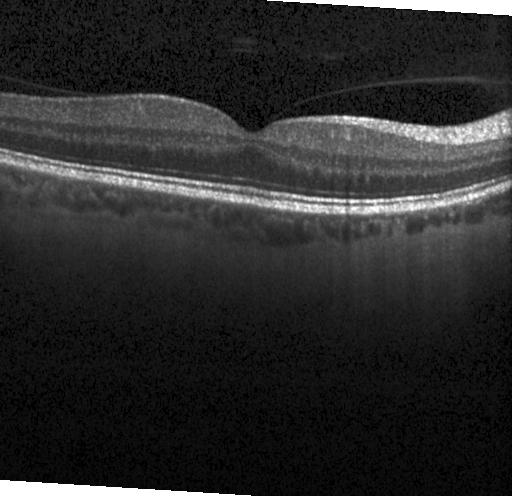
Acquired on a Heidelberg Spectralis; through the macula; OCT line scan; spectral-domain optical coherence tomography. Impression: no evidence of choroidal neovascularization, diabetic macular edema, or drusen.